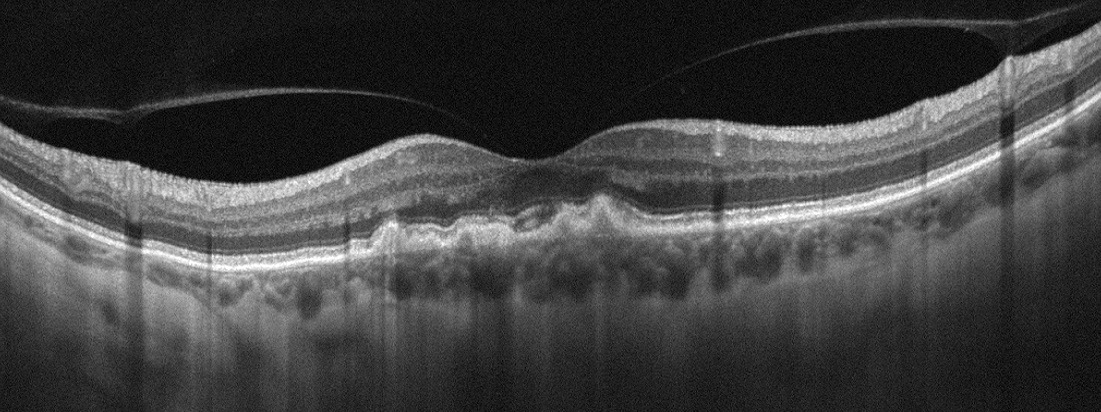

This B-scan demonstrates age-related macular degeneration.